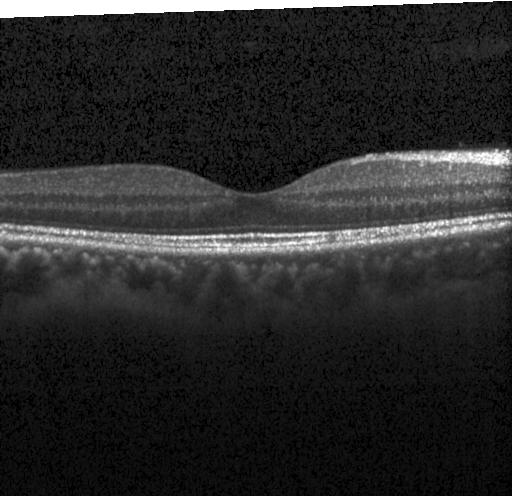

Centered on the fovea · spectral-domain optical coherence tomography · retinal OCT B-scan · instrument: Heidelberg Spectralis
OCT finding: no choroidal neovascularization, no diabetic macular edema, and no drusen.